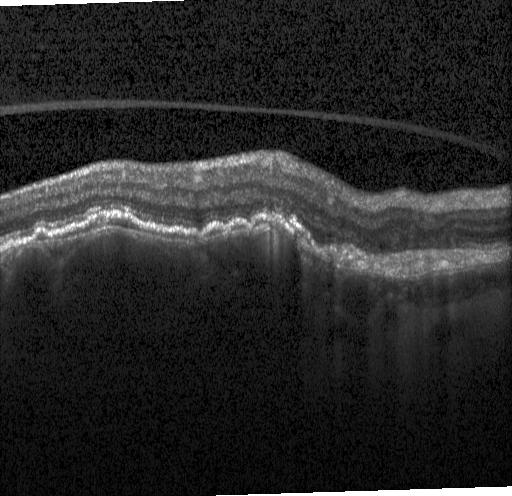
Instrument: Heidelberg Spectralis. Retinal OCT B-scan. Spectral-domain OCT.
Macular OCT: a choroidal neovascular membrane.